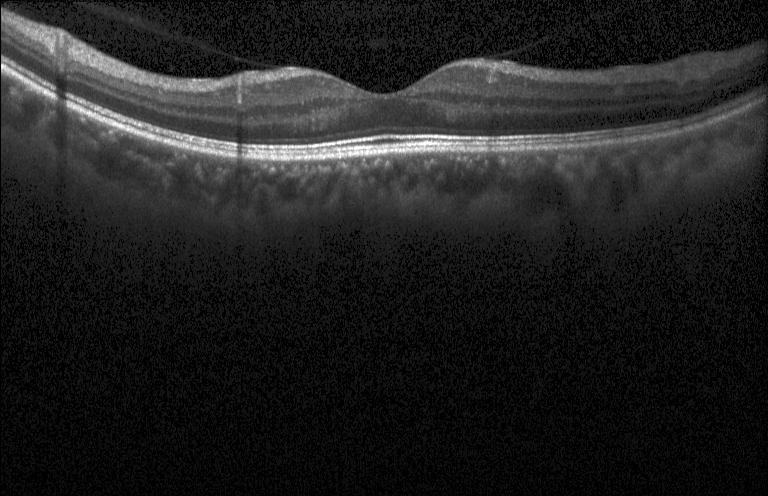

OCT finding: no choroidal neovascularization, diabetic macular edema, or drusen.